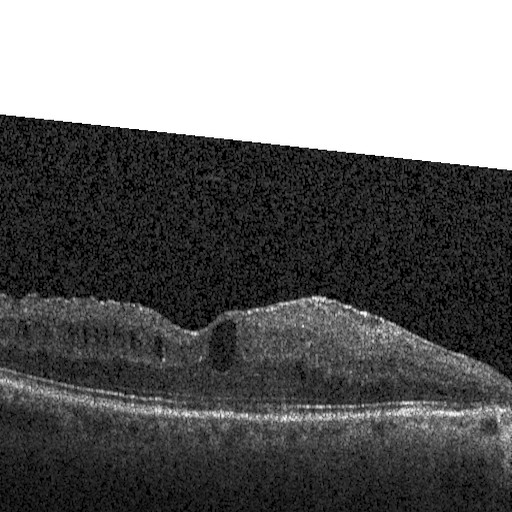 Retinal OCT cross-section showing DME.